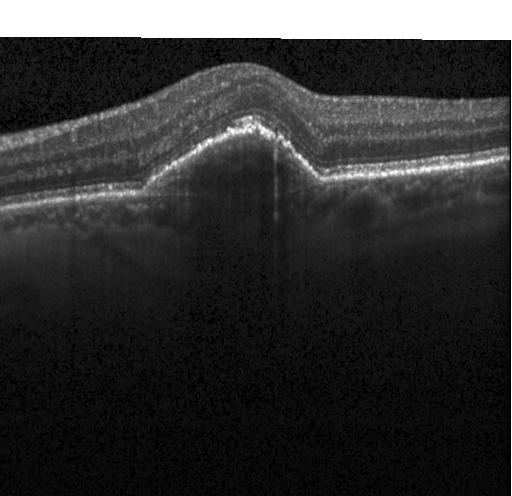 The scan shows a choroidal neovascular membrane.